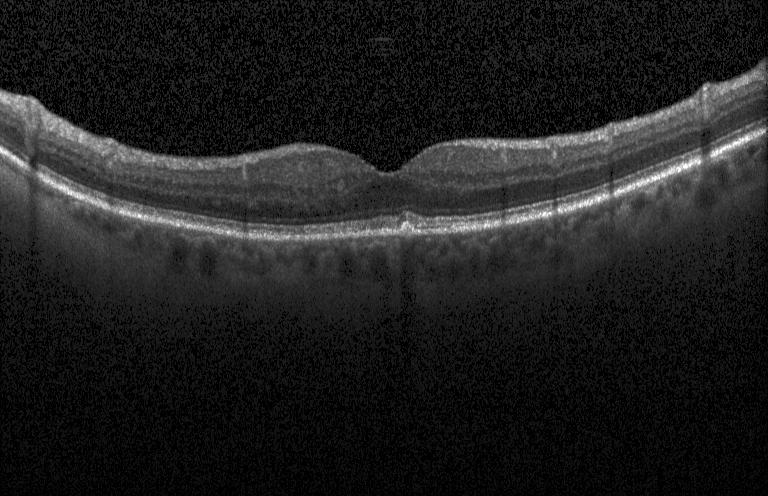 Retinal OCT B-scan. Finding: drusen.